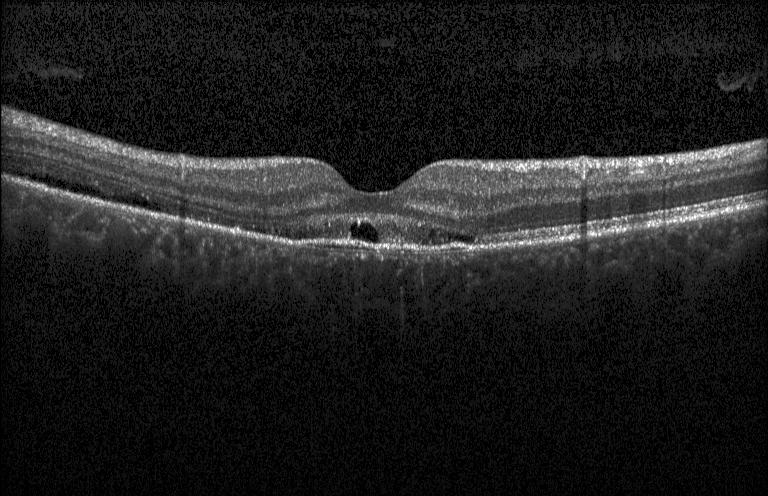

Retinal OCT B-scan — Finding: a choroidal neovascular membrane.